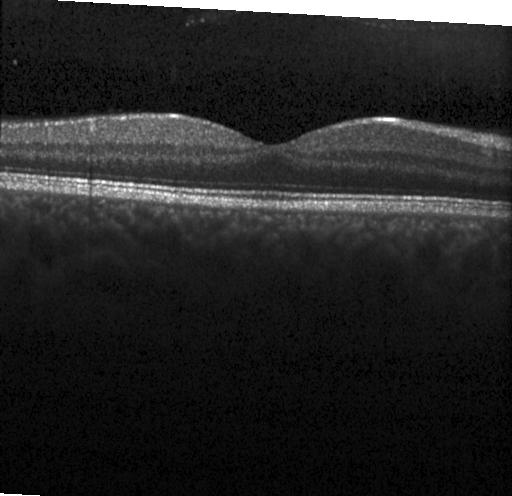

Impression: no CNV, no DME, and no drusen.